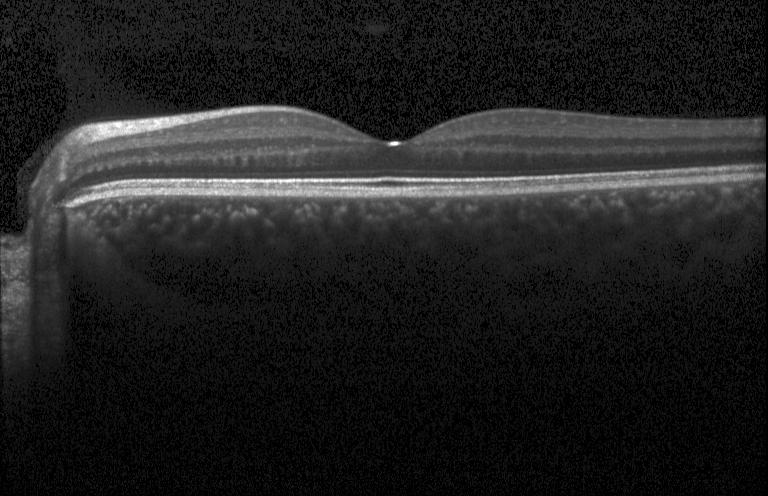

Macular OCT demonstrating no choroidal neovascularization, diabetic macular edema, or drusen.